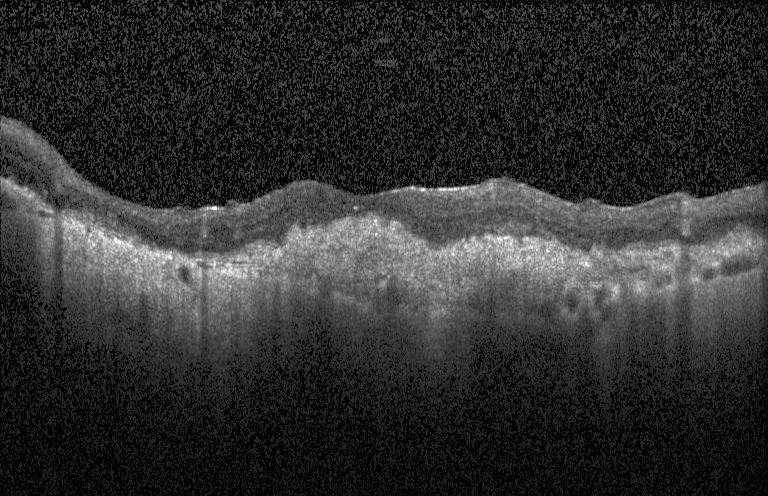
OCT line scan, macular scan, acquired on a Heidelberg Spectralis
Dx: choroidal neovascularization.